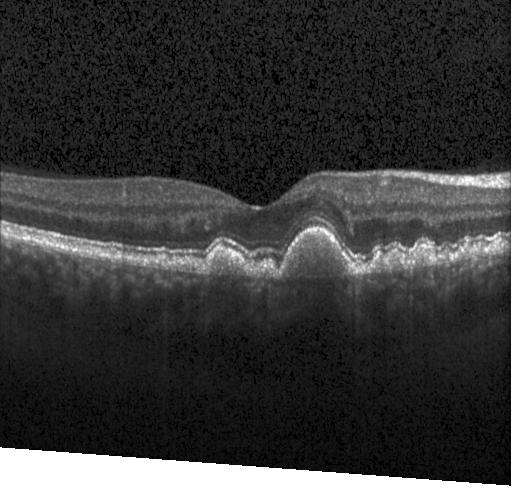 Heidelberg Spectralis; SD-OCT; centered on the fovea; retinal OCT cross-section.
Multiple drusen.